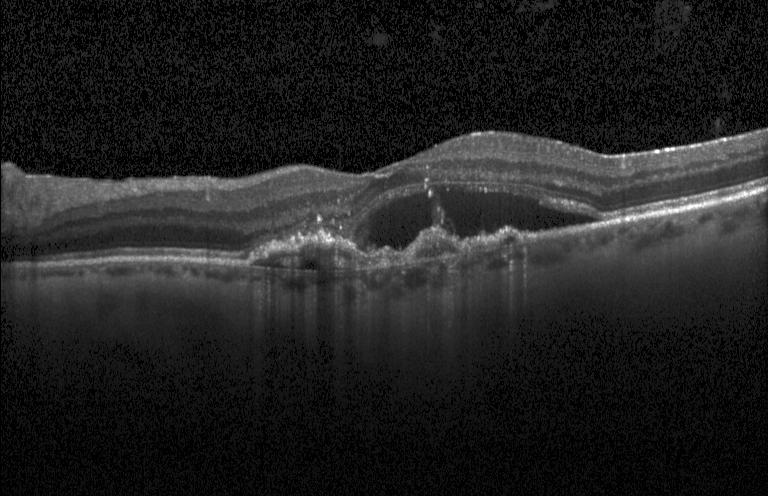 Retinal OCT cross-section, centered on the fovea, Heidelberg Spectralis — Assessment: a choroidal neovascular membrane.